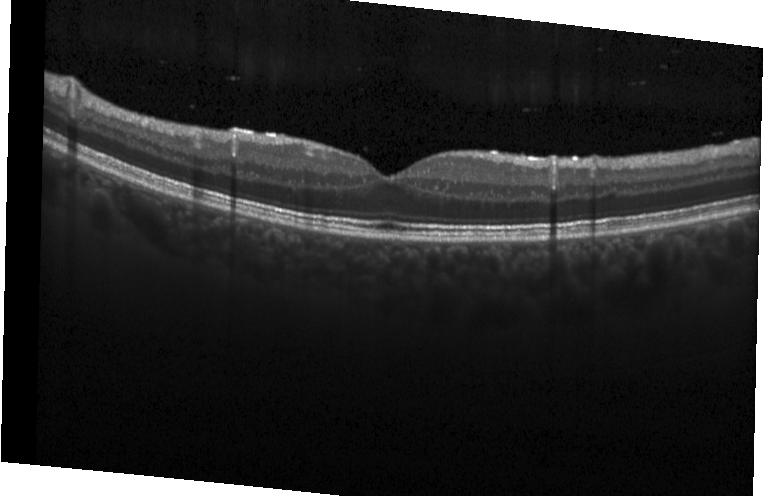
Through the macula · optical coherence tomography scan — No choroidal neovascularization, diabetic macular edema, or drusen.